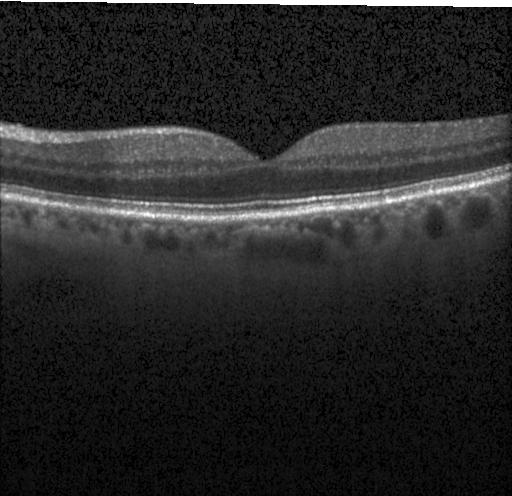 OCT line scan; macular scan
This B-scan demonstrates no CNV, no DME, and no drusen.